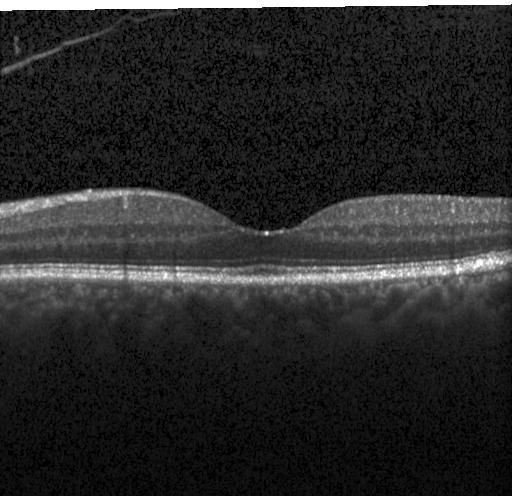 Retinal OCT B-scan, macular scan. Diagnosis: no choroidal neovascularization, diabetic macular edema, or drusen.